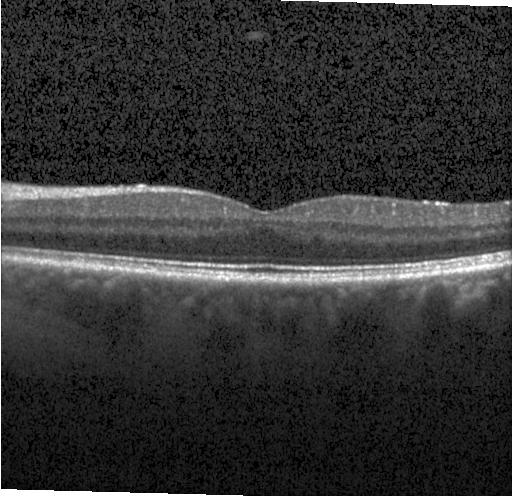

Spectral-domain optical coherence tomography. Acquired on a Heidelberg Spectralis. Optical coherence tomography B-scan. Through the macula. Impression: neither CNV, DME, nor drusen.